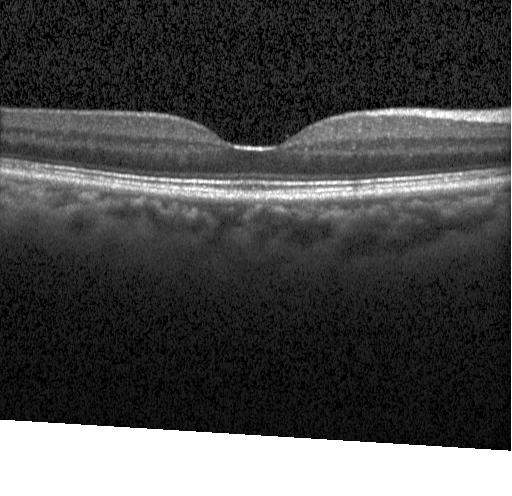

Horizontal scan through the fovea. Heidelberg Spectralis. Spectral-domain OCT. OCT B-scan — Finding: no evidence of choroidal neovascularization, diabetic macular edema, or drusen.